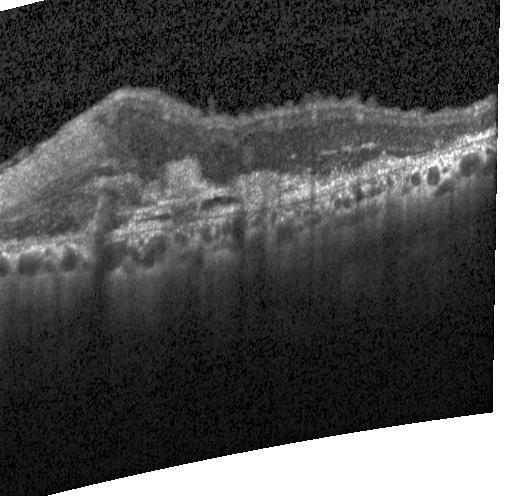
The scan shows choroidal neovascularization (CNV).